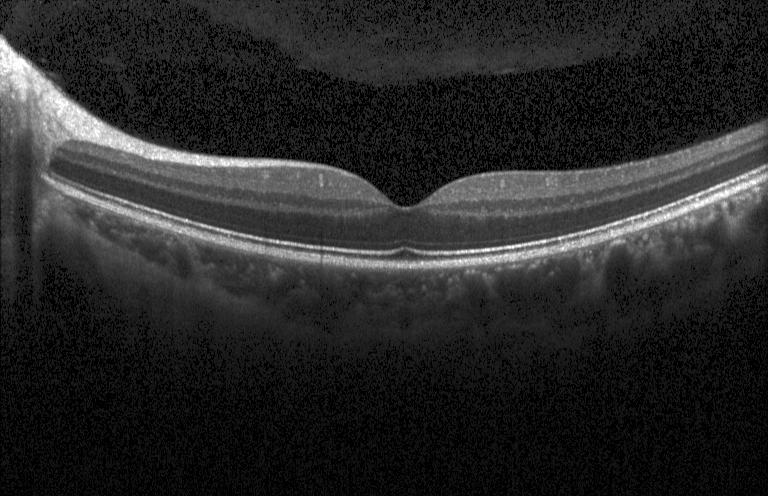 Finding: no CNV, DME, or drusen.